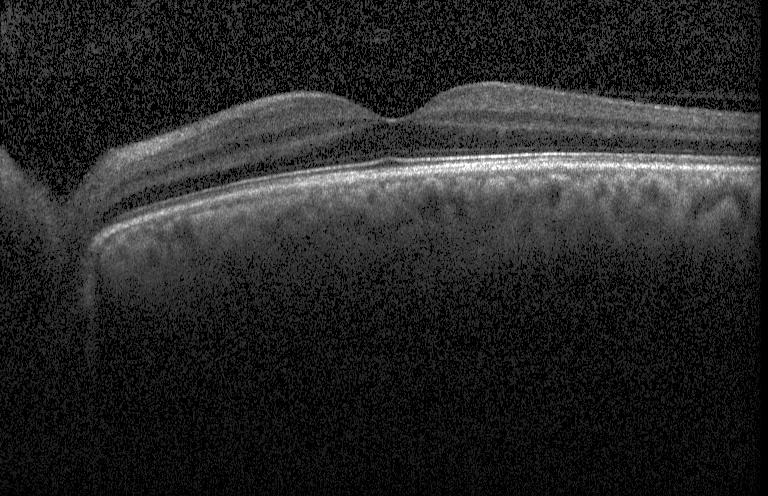

Diagnosis: no evidence of CNV, DME, or drusen.